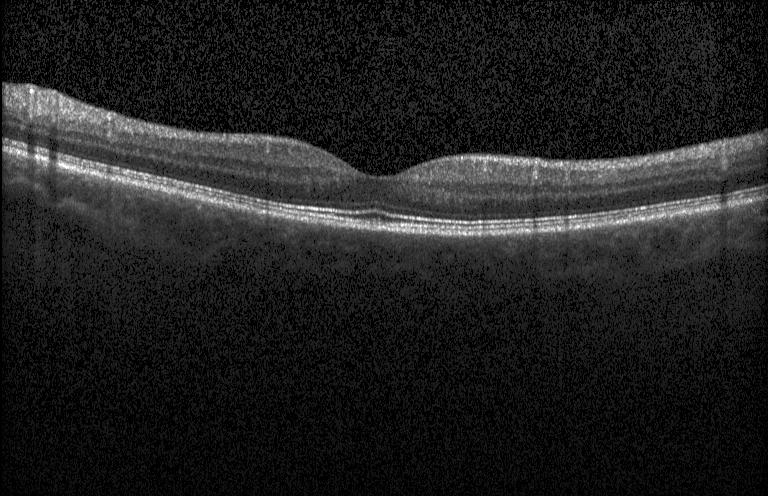 Centered on the fovea; SD-OCT; optical coherence tomography B-scan; Heidelberg Spectralis. The scan shows no choroidal neovascularization, no diabetic macular edema, and no drusen.